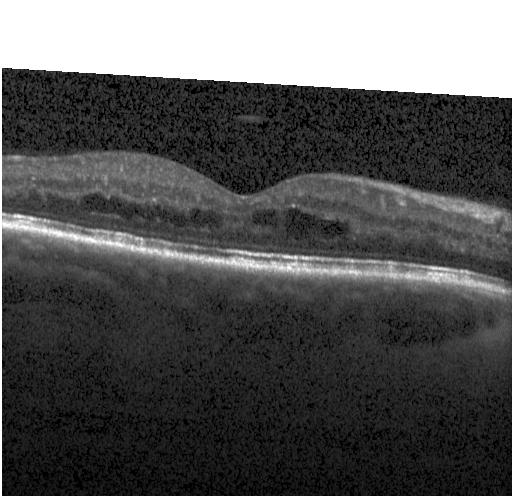 OCT line scan.
DME.